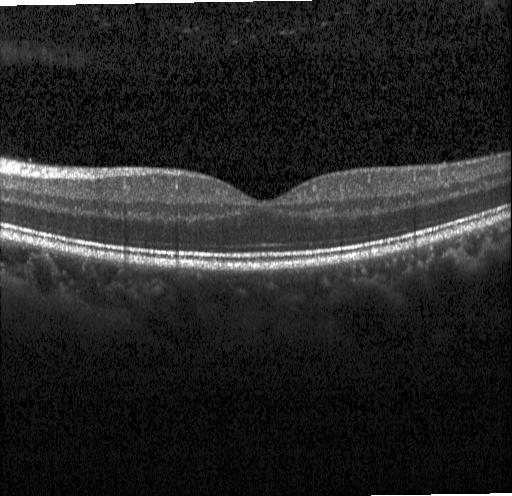
Retinal OCT cross-section. Finding: no choroidal neovascularization, no diabetic macular edema, and no drusen.